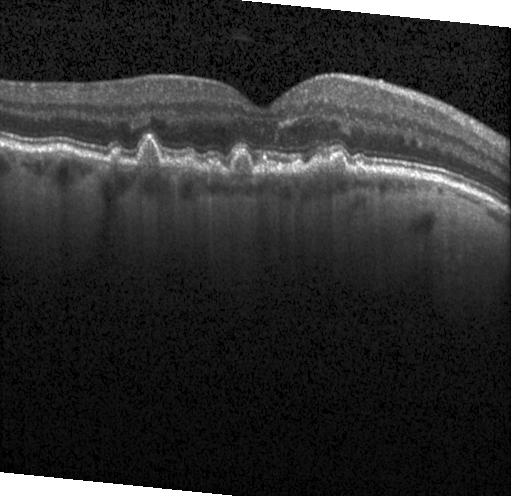
Spectral-domain OCT B-scan: multiple drusen.